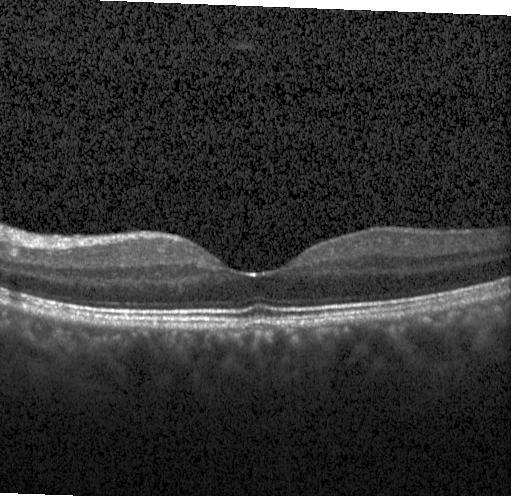 Impression: no choroidal neovascularization, diabetic macular edema, or drusen.